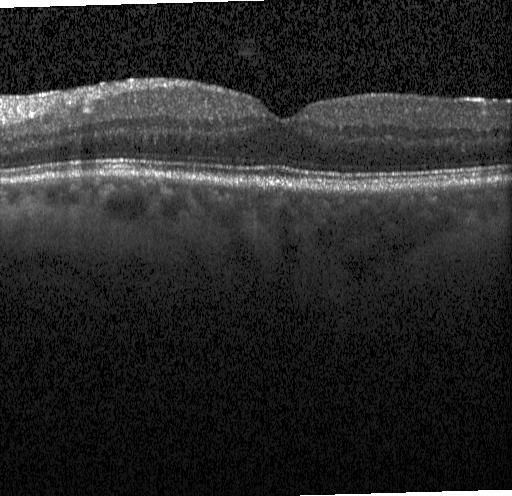

OCT B-scan.
Finding: neither choroidal neovascularization, diabetic macular edema, nor drusen.